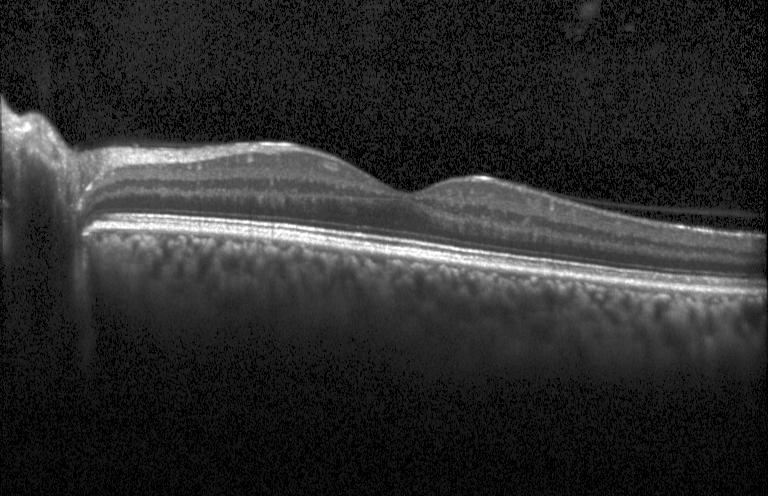
OCT finding: no choroidal neovascularization, no diabetic macular edema, and no drusen.